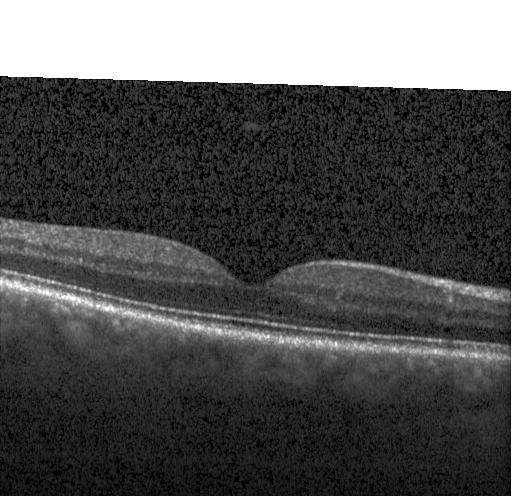

Dx: no evidence of choroidal neovascularization, diabetic macular edema, or drusen.